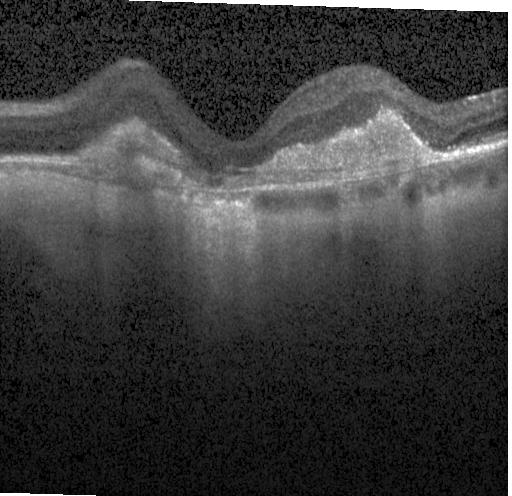
Dx: a choroidal neovascular membrane.